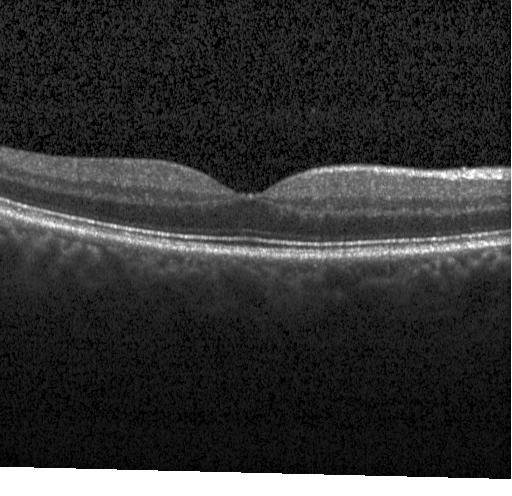

The scan shows no choroidal neovascularization, no diabetic macular edema, and no drusen.